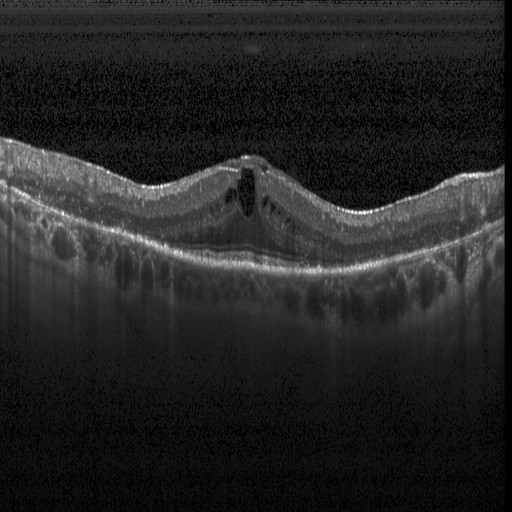 Horizontal scan through the fovea, optical coherence tomography B-scan, spectral-domain OCT, Heidelberg Spectralis OCT system.
Impression: DME.